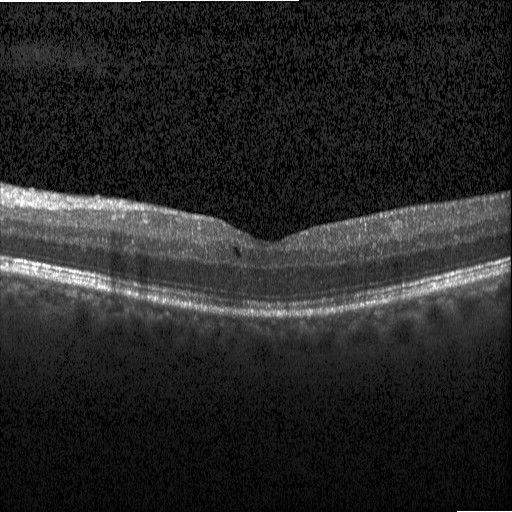
Finding: diabetic macular edema (DME).